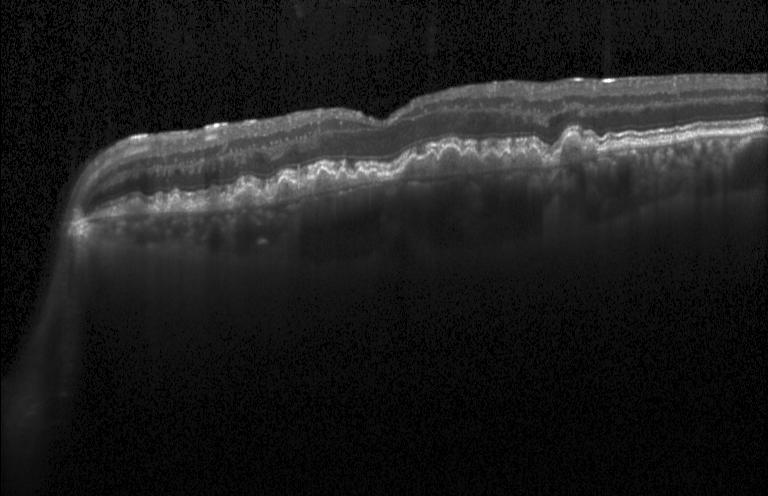
Retinal OCT cross-section, spectral-domain OCT — Finding: a choroidal neovascular membrane.